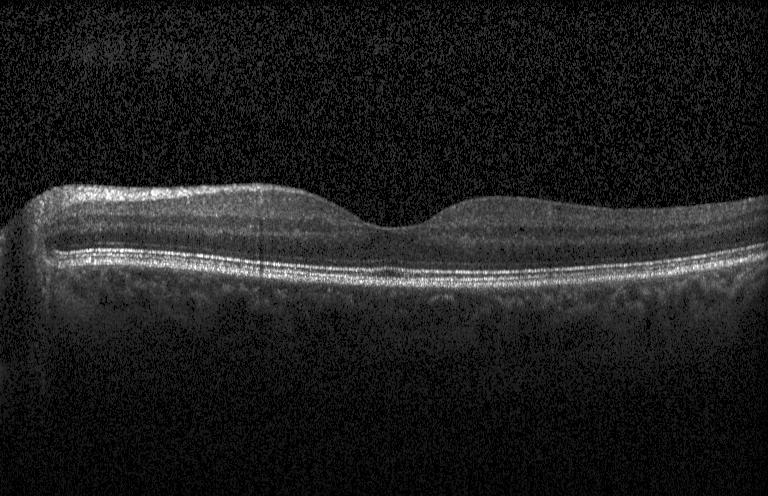 Retinal OCT cross-section — Diagnosis: neither choroidal neovascularization, diabetic macular edema, nor drusen.